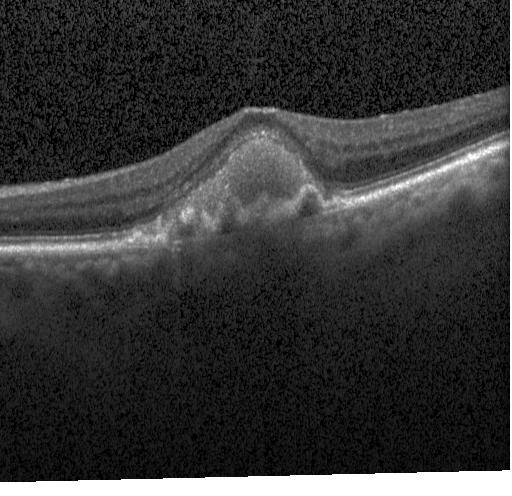
Finding: a choroidal neovascular membrane.